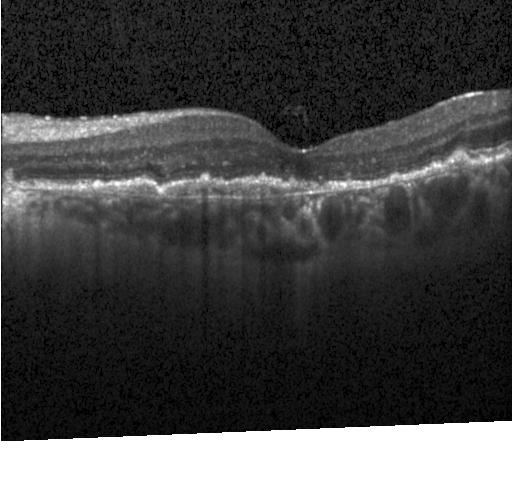 Optical coherence tomography scan · macular scan · spectral-domain optical coherence tomography · Heidelberg Spectralis OCT system
Assessment: CNV.